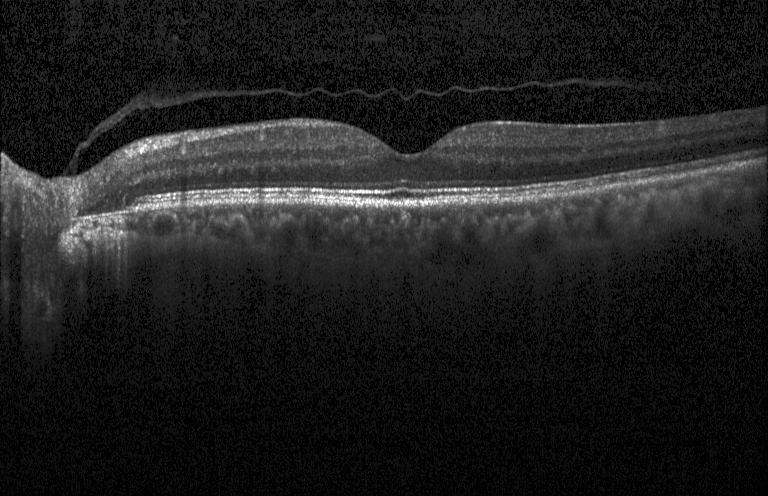

Retinal OCT cross-section showing no evidence of choroidal neovascularization, diabetic macular edema, or drusen.